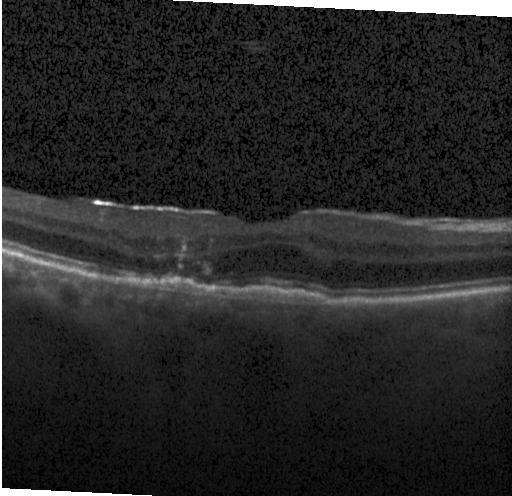
Retinal OCT cross-section. Instrument: Heidelberg Spectralis. Impression: a choroidal neovascular membrane.